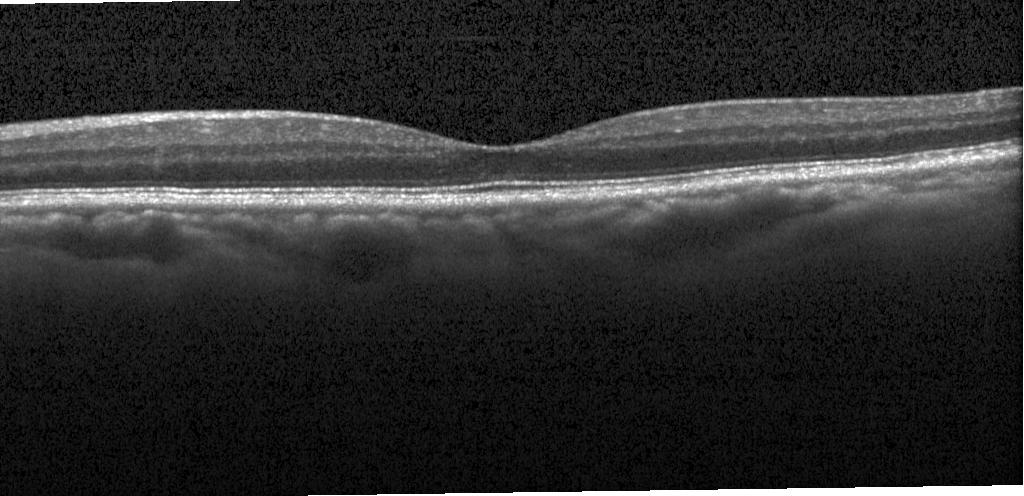
Fovea-centered; SD-OCT; OCT B-scan. Dx: no choroidal neovascularization, no diabetic macular edema, and no drusen.